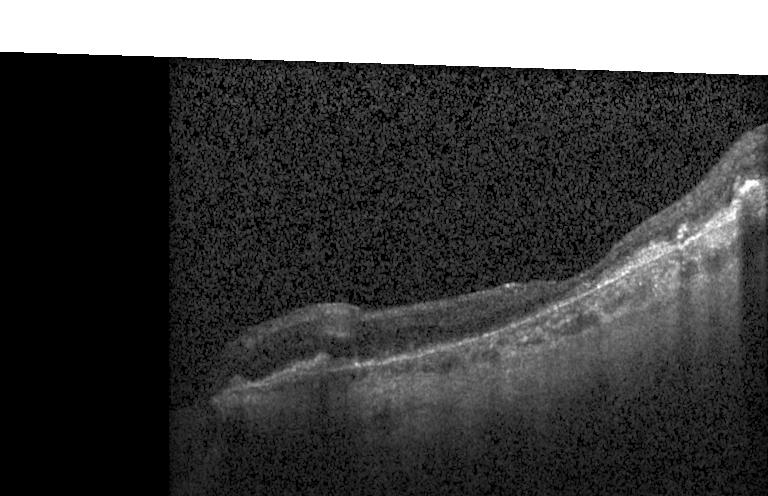

Acquired on a Heidelberg Spectralis, retinal OCT cross-section — Assessment: a choroidal neovascular membrane.